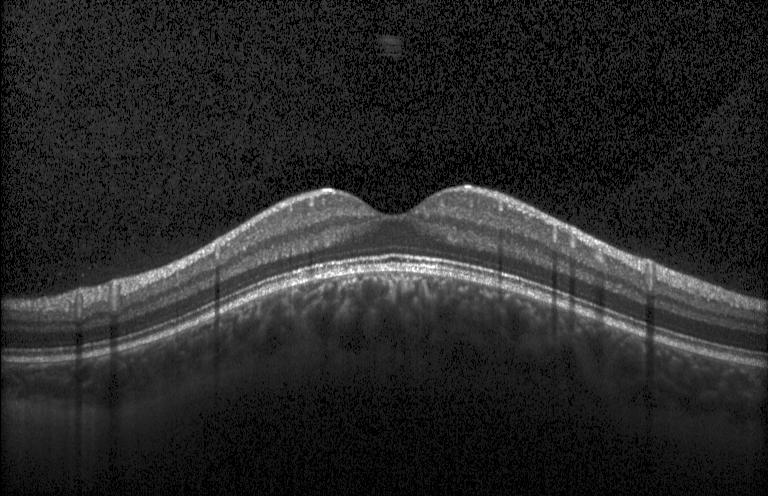
Diagnosis: no evidence of CNV, DME, or drusen.